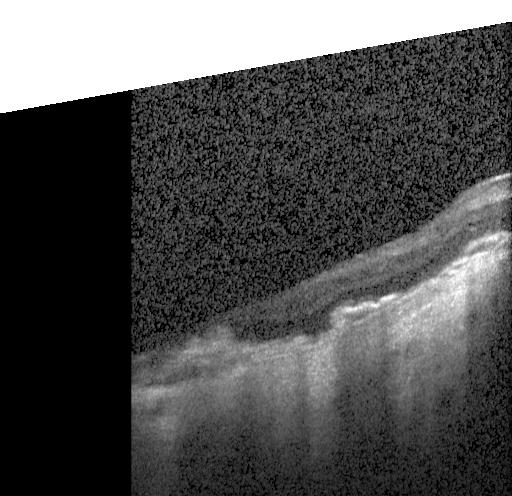 Retinal OCT cross-section showing choroidal neovascularization (CNV).